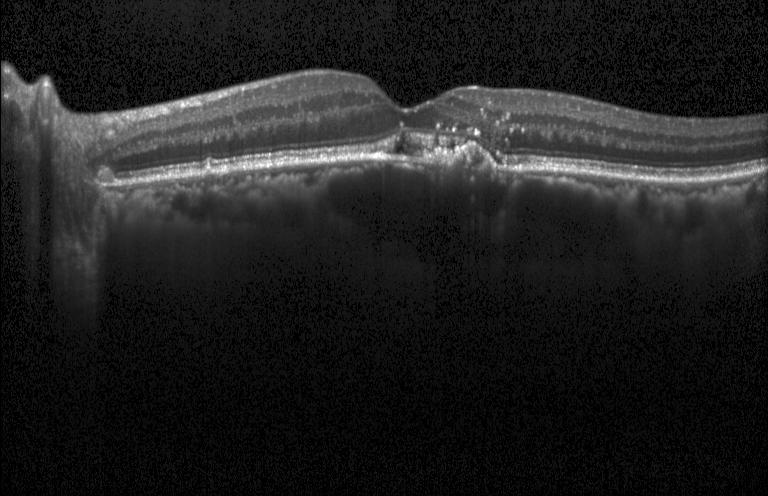

OCT scan showing a choroidal neovascular membrane.